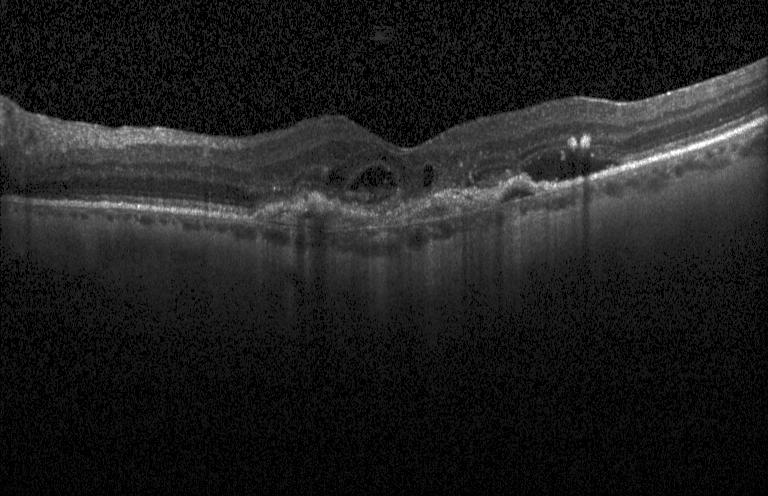 Impression: CNV.